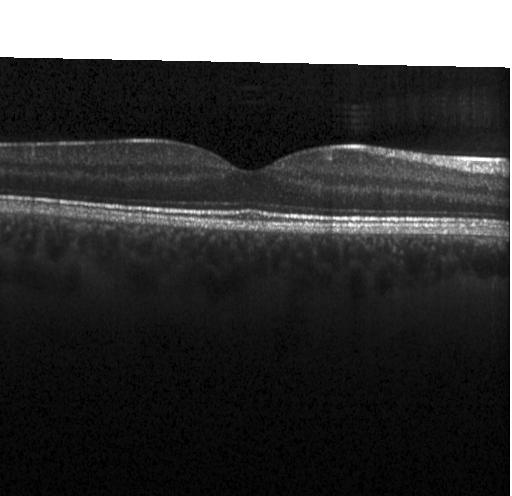 Macular OCT: no CNV, DME, or drusen.